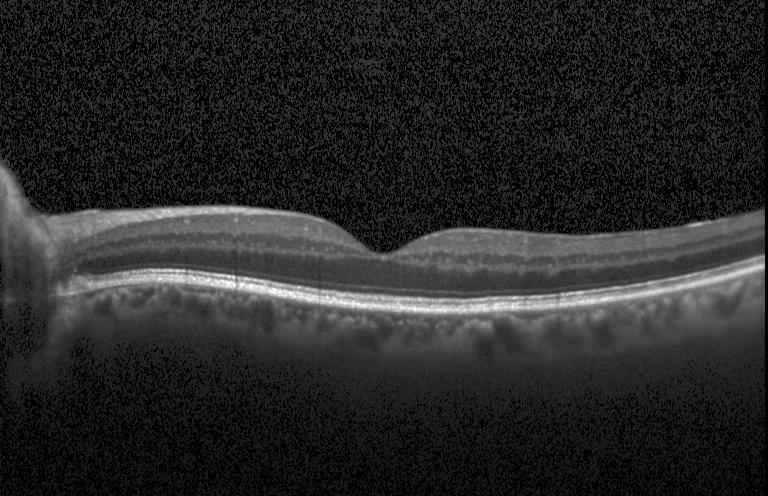 Dx: neither choroidal neovascularization, diabetic macular edema, nor drusen.